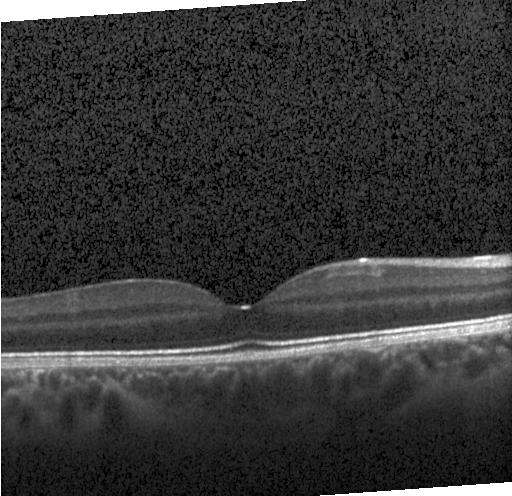 Dx: no evidence of choroidal neovascularization, diabetic macular edema, or drusen.